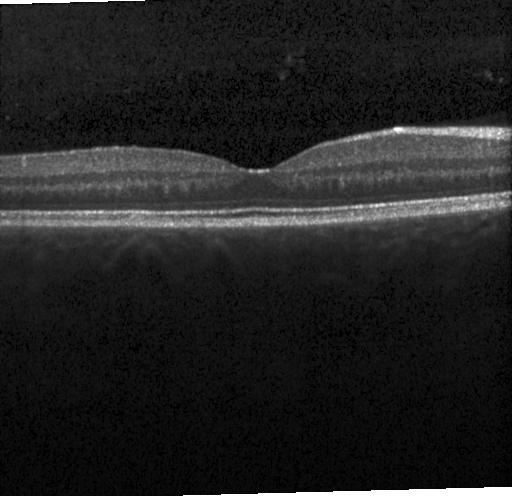 Retinal OCT cross-section.
Dx: no evidence of CNV, DME, or drusen.